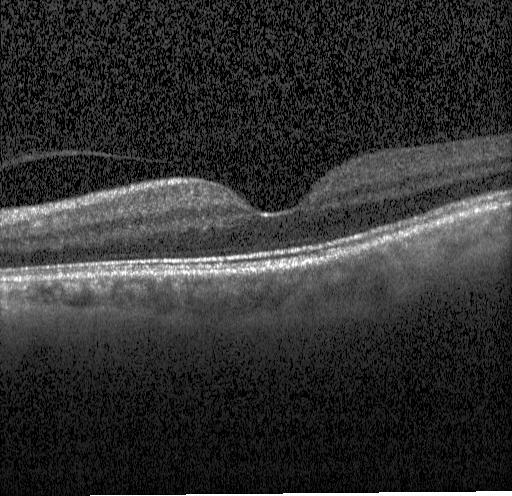

OCT scan showing no CNV, no DME, and no drusen.